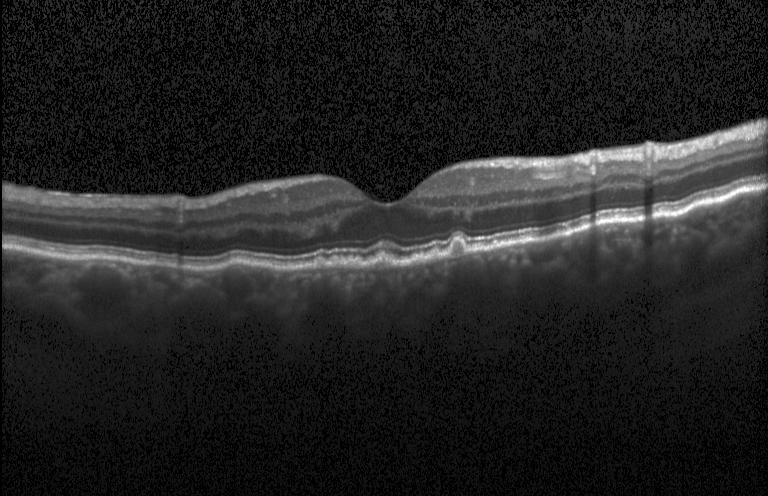
Spectral-domain OCT B-scan: multiple drusen.